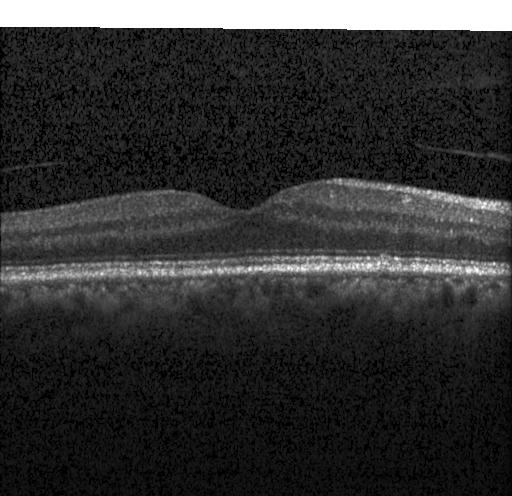

Retinal OCT B-scan, through the macula, acquired on a Heidelberg Spectralis
Dx: neither choroidal neovascularization, diabetic macular edema, nor drusen.